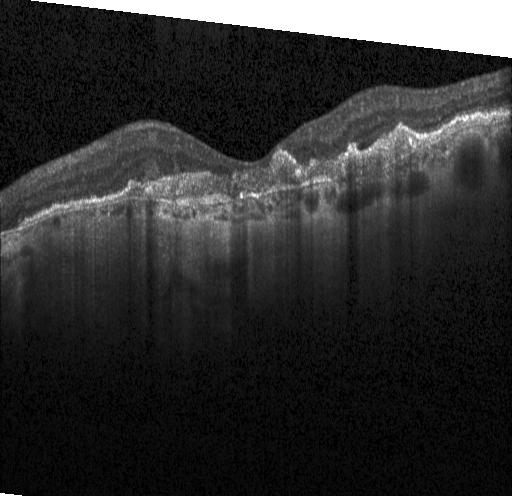 OCT finding: choroidal neovascularization.